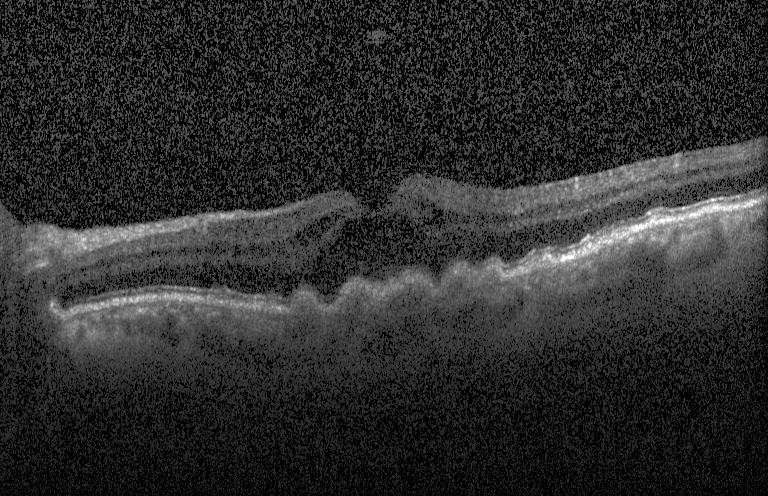
OCT B-scan
Impression: drusen.